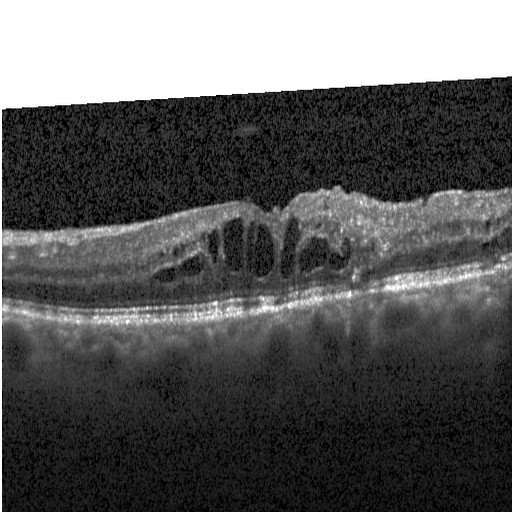

OCT B-scan · fovea-centered · instrument: Heidelberg Spectralis · spectral-domain optical coherence tomography
Macular OCT: diabetic macular edema.